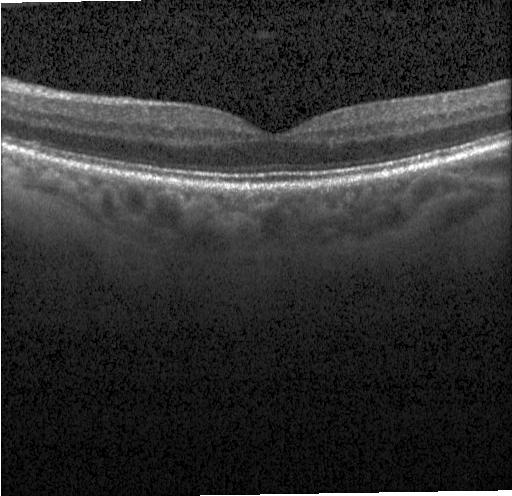 Retinal OCT cross-section. Impression: no evidence of choroidal neovascularization, diabetic macular edema, or drusen.